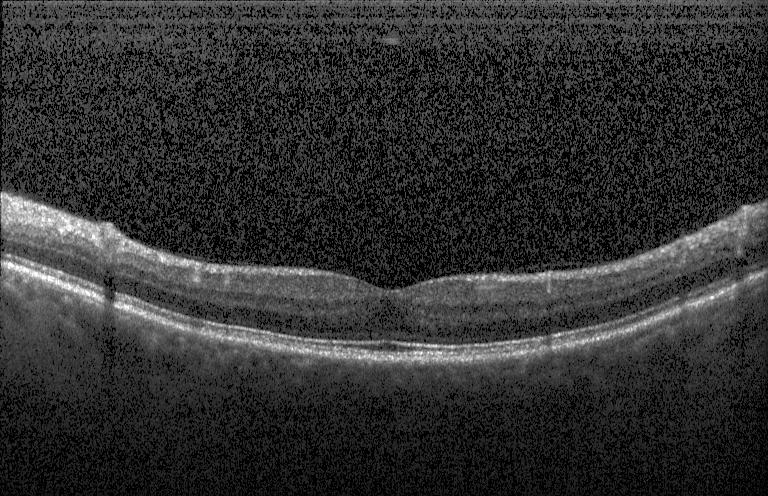

Horizontal scan through the fovea, retinal OCT B-scan. Impression: no choroidal neovascularization, diabetic macular edema, or drusen.